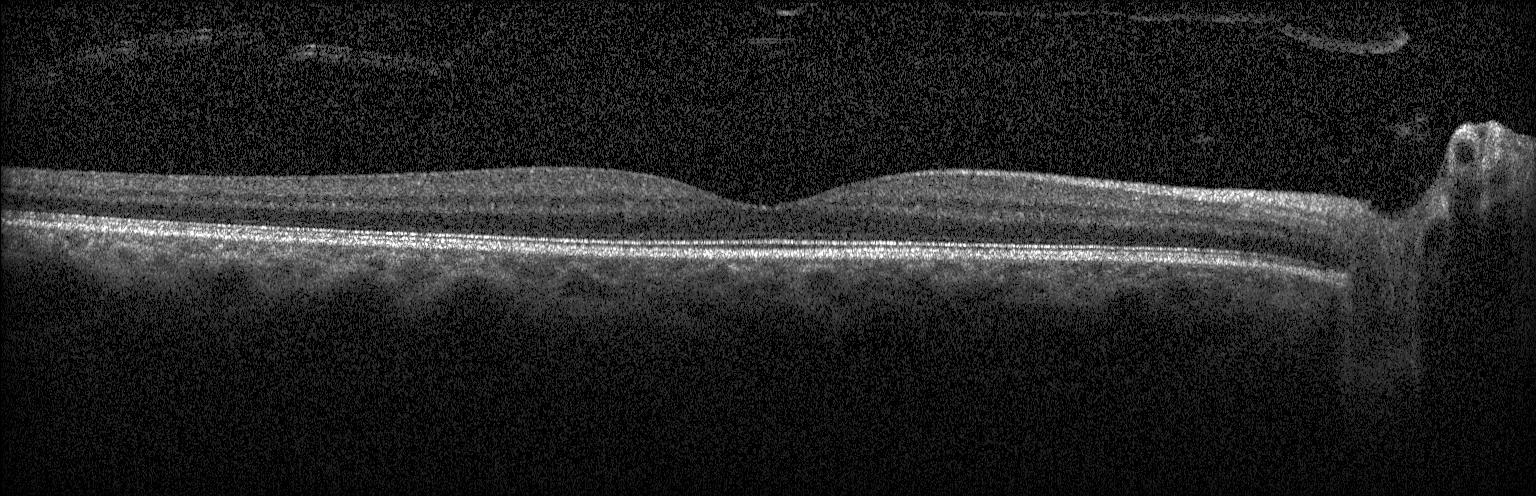 The scan shows no evidence of choroidal neovascularization, diabetic macular edema, or drusen.